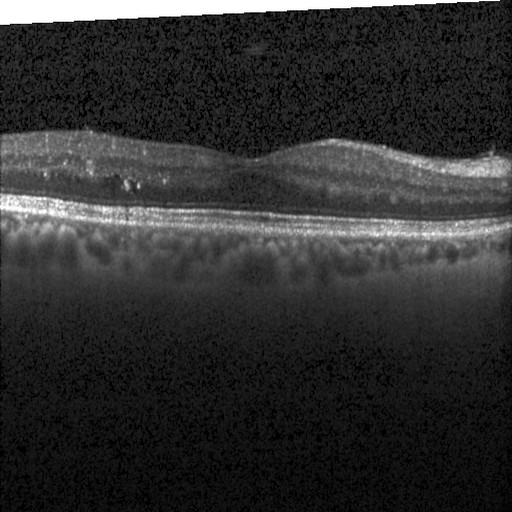

OCT B-scan
Assessment: diabetic macular edema.